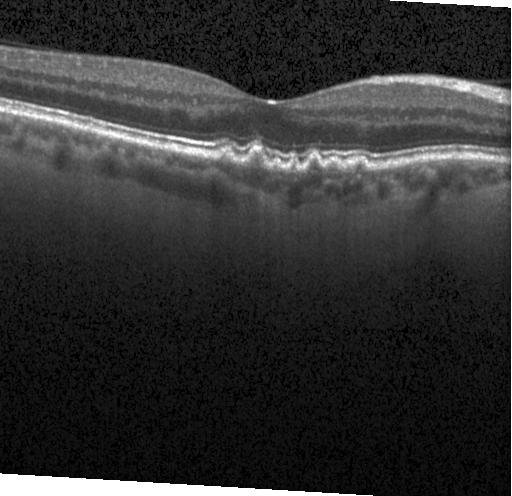

Macular OCT demonstrating drusen.